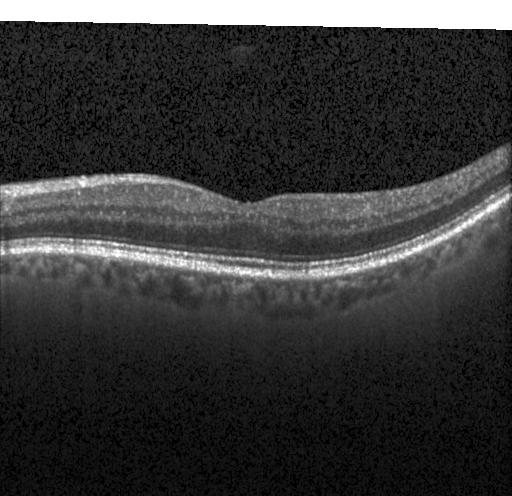

Macular OCT: neither CNV, DME, nor drusen.